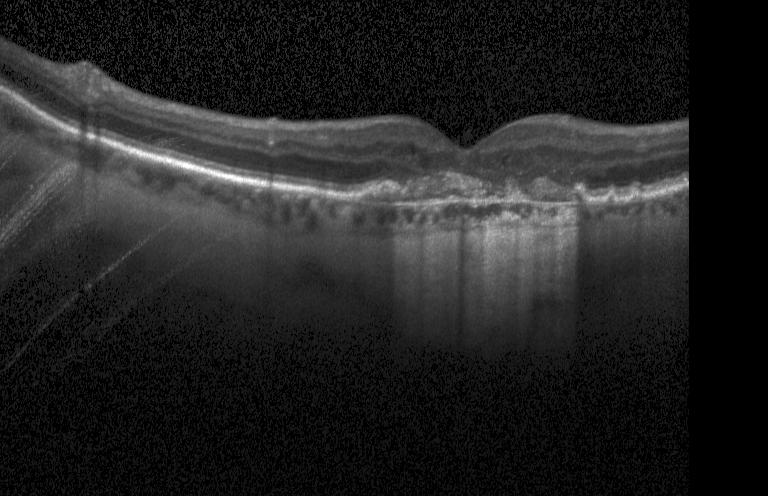
Acquired on a Heidelberg Spectralis; retinal OCT B-scan. The scan shows choroidal neovascularization (CNV).